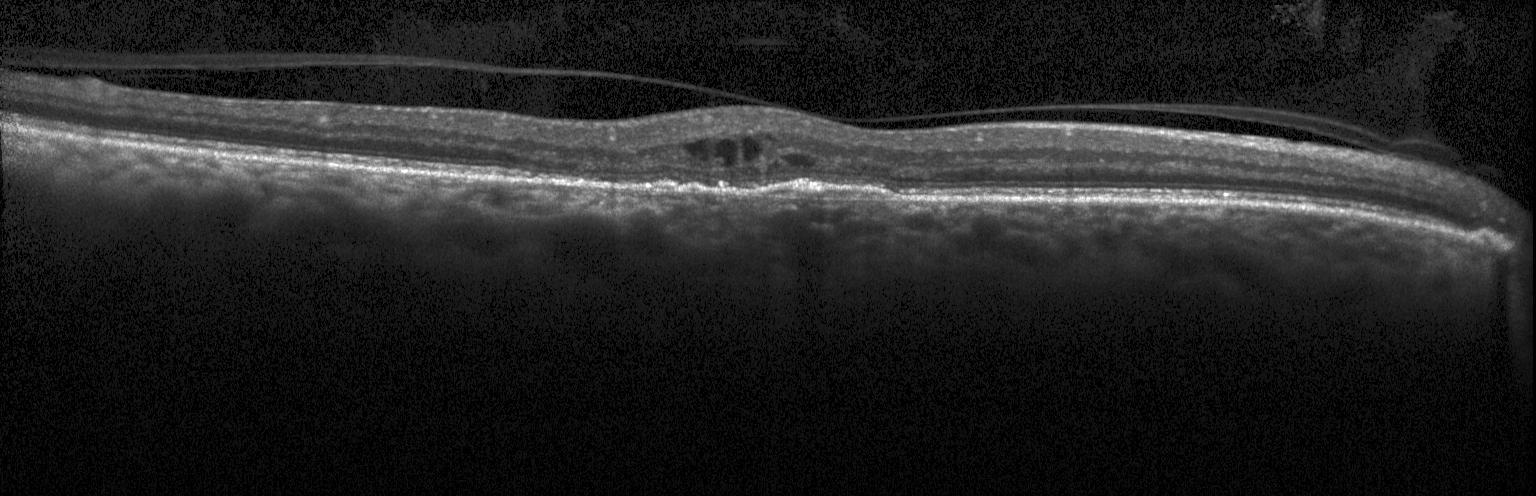 Spectral-domain OCT B-scan: a choroidal neovascular membrane.